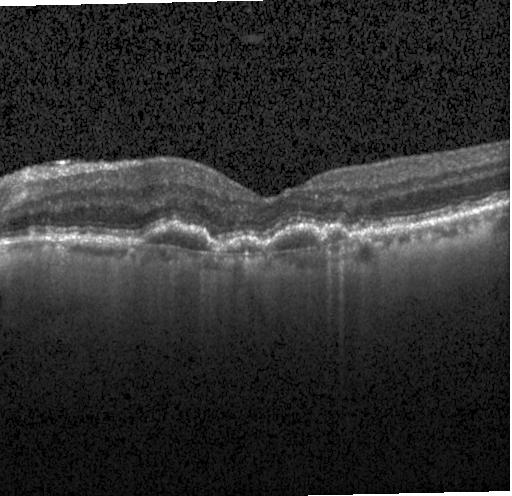

Retinal OCT B-scan. Through the macula.
Assessment: a choroidal neovascular membrane.